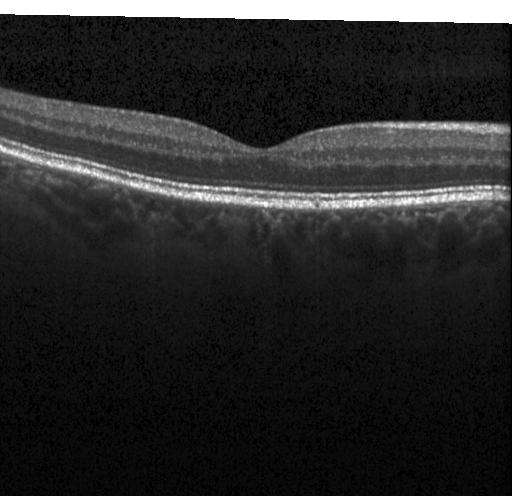

Heidelberg Spectralis · retinal OCT B-scan · spectral-domain OCT · macular scan.
Macular OCT: no choroidal neovascularization, diabetic macular edema, or drusen.